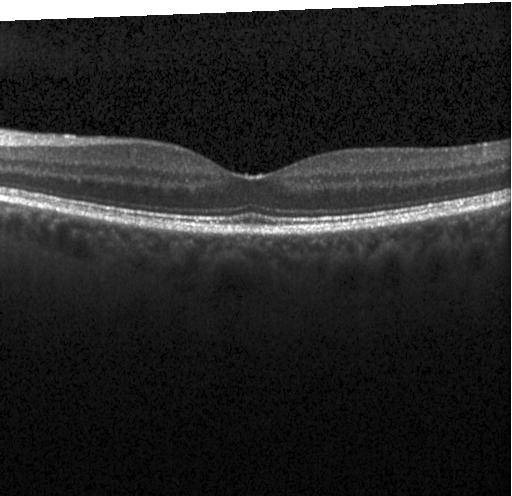 Optical coherence tomography B-scan. Fovea-centered. SD-OCT
Impression: no evidence of CNV, DME, or drusen.